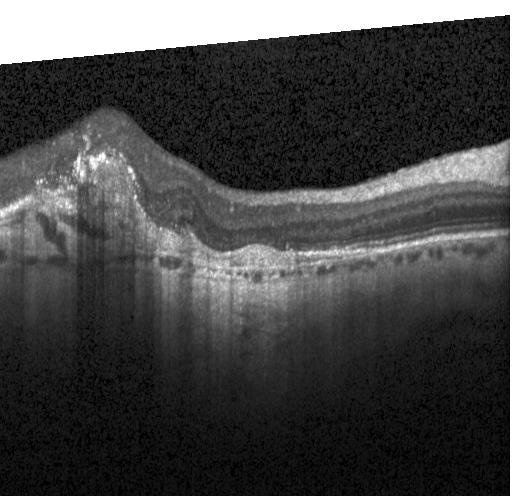

Impression: a choroidal neovascular membrane.